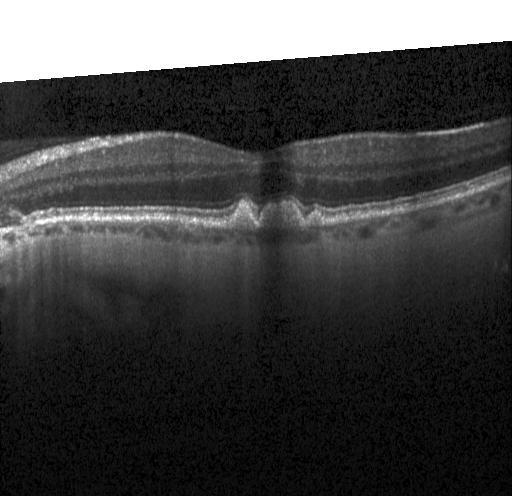

OCT line scan. Diagnosis: multiple drusen.